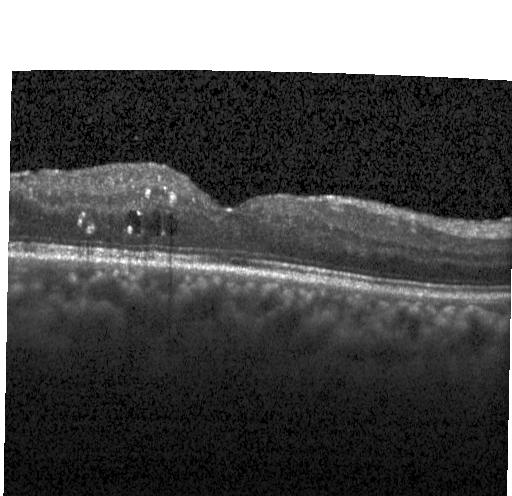
SD-OCT · fovea-centered · optical coherence tomography B-scan.
Impression: diabetic macular edema (DME).